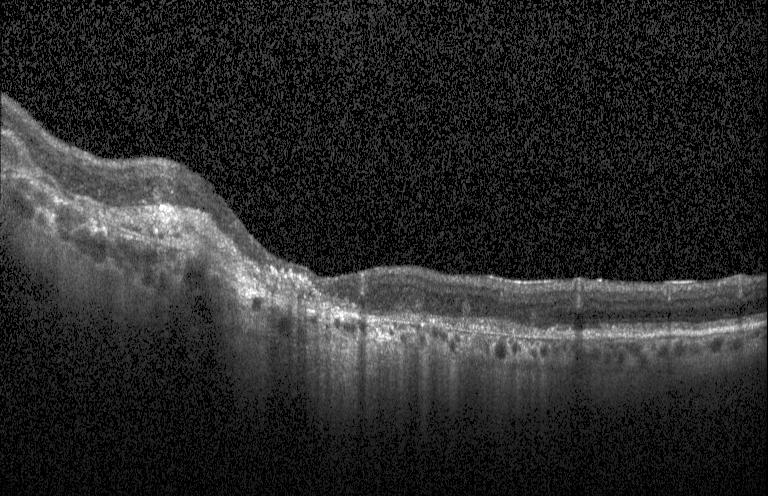

Macular OCT: CNV.